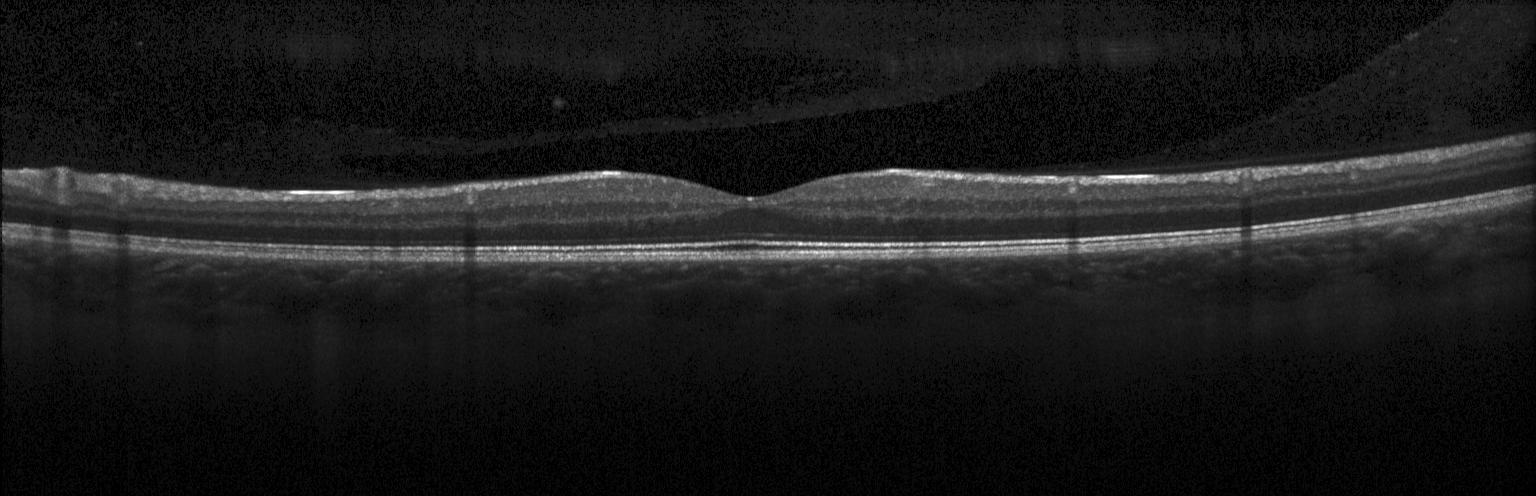
Centered on the fovea · retinal OCT B-scan — Dx: no evidence of CNV, DME, or drusen.